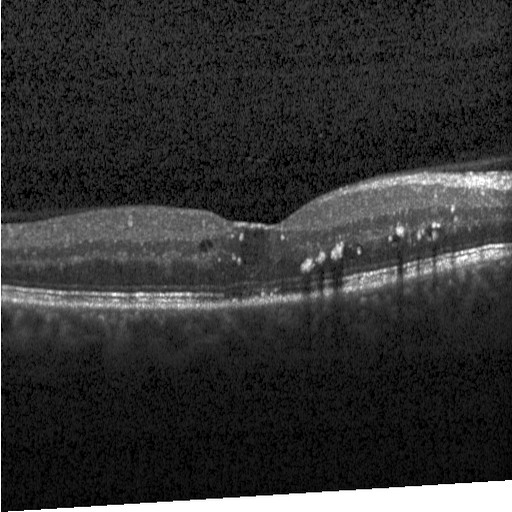
OCT line scan · spectral-domain OCT — The scan shows DME.